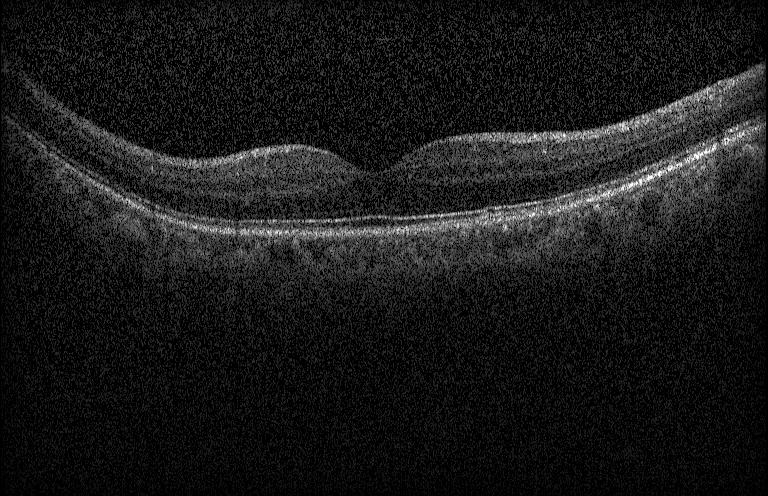 Optical coherence tomography B-scan.
Neither choroidal neovascularization, diabetic macular edema, nor drusen.